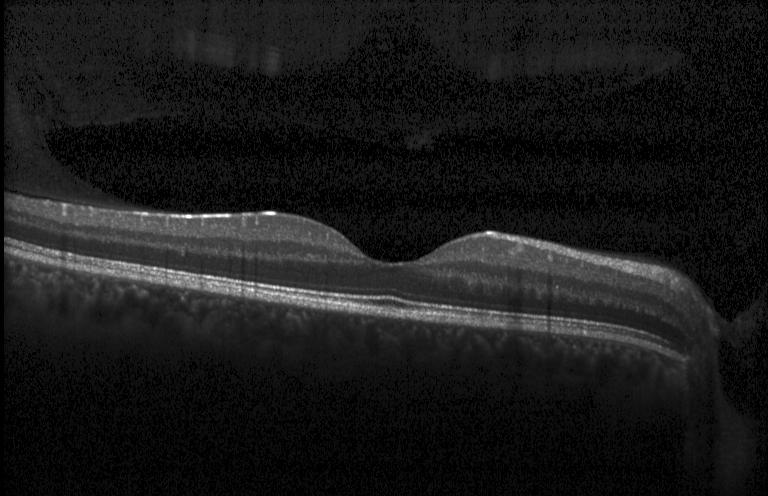 Heidelberg Spectralis. Fovea-centered. OCT B-scan — Macular OCT: no choroidal neovascularization, diabetic macular edema, or drusen.